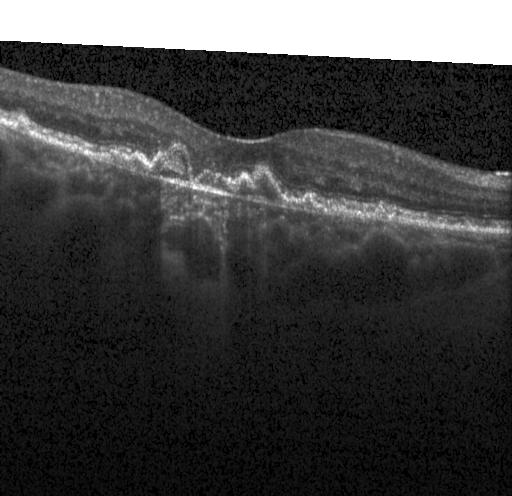
SD-OCT; acquired on a Heidelberg Spectralis; OCT B-scan; through the macula — OCT finding: choroidal neovascularization.